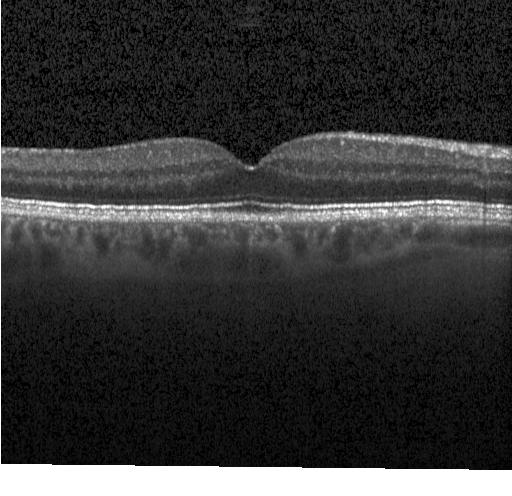
Heidelberg Spectralis · spectral-domain optical coherence tomography · through the macula · retinal OCT cross-section — Impression: no CNV, no DME, and no drusen.